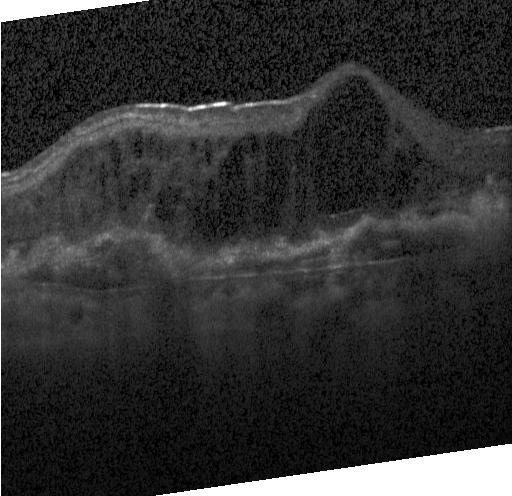 OCT B-scan, Heidelberg Spectralis.
OCT finding: a choroidal neovascular membrane.